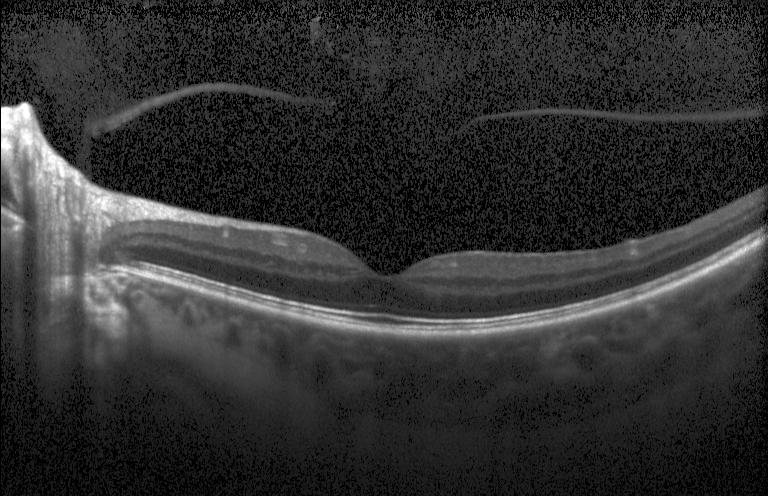
OCT B-scan; macular scan; SD-OCT.
Diagnosis: no CNV, no DME, and no drusen.